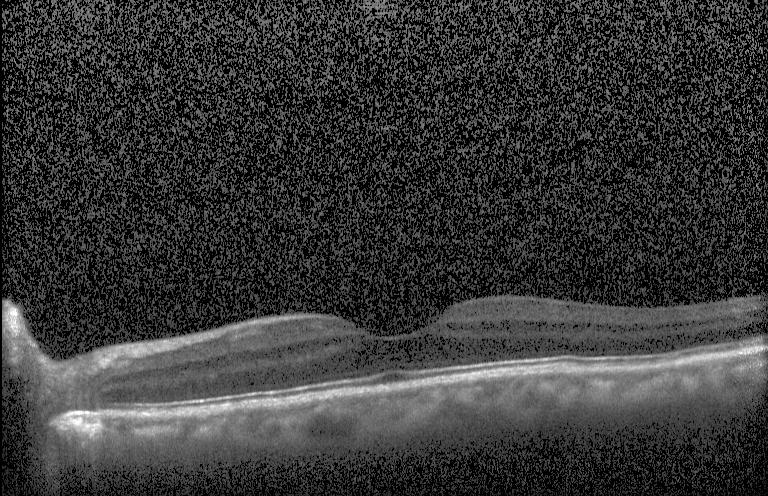 OCT B-scan showing neither choroidal neovascularization, diabetic macular edema, nor drusen.